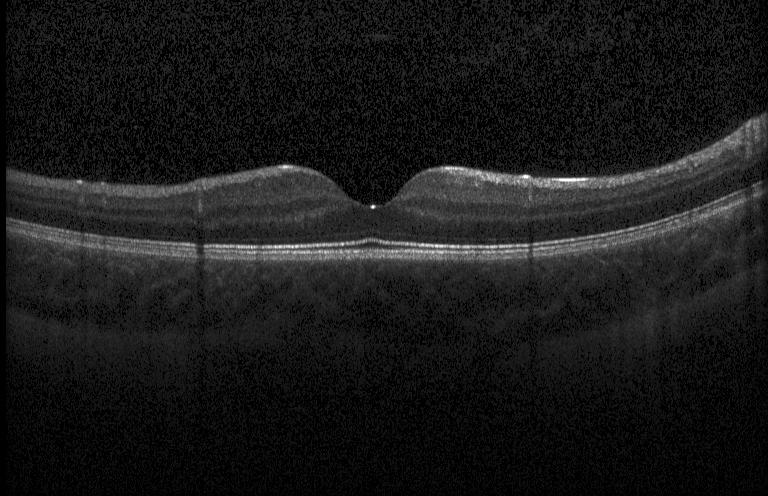 OCT line scan, spectral-domain optical coherence tomography. Impression: no choroidal neovascularization, no diabetic macular edema, and no drusen.